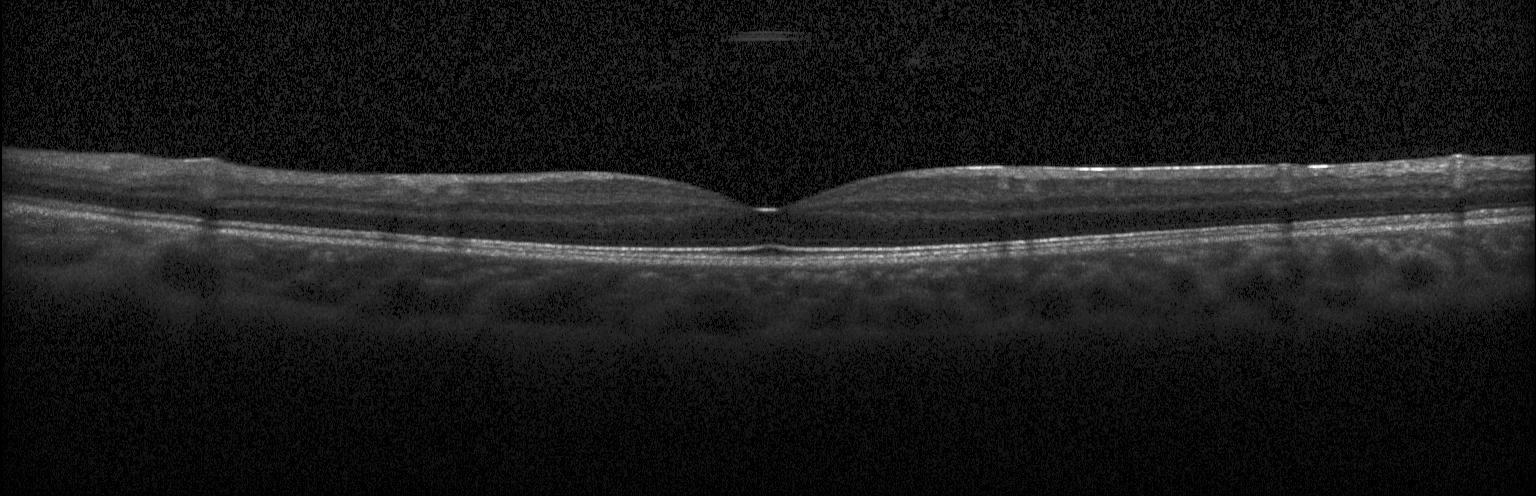 Optical coherence tomography scan — This B-scan demonstrates no CNV, DME, or drusen.